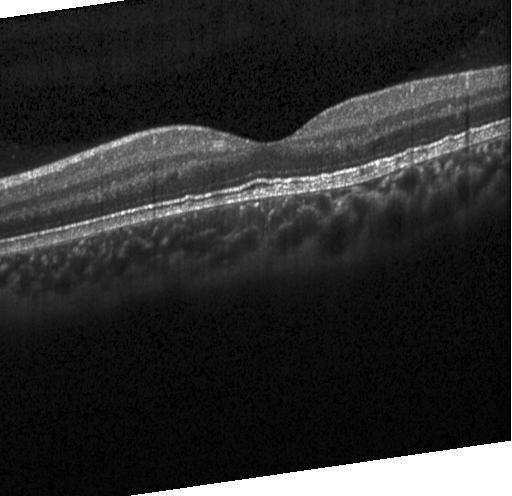 OCT B-scan showing no CNV, DME, or drusen.